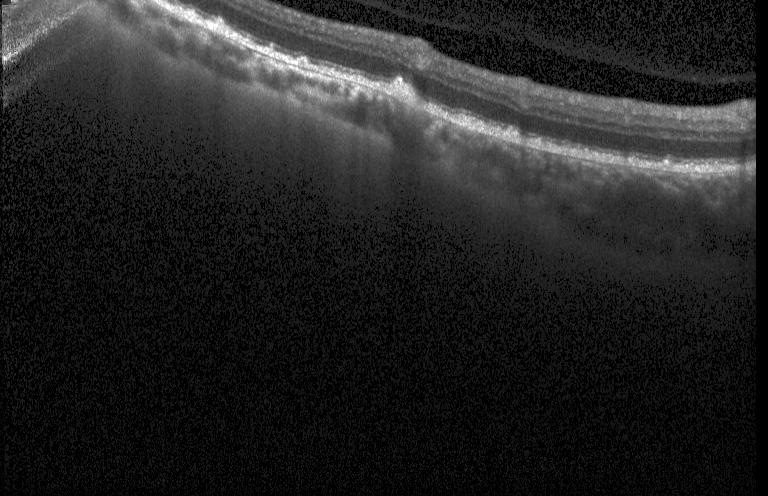

Macular scan. OCT B-scan — Finding: multiple drusen.